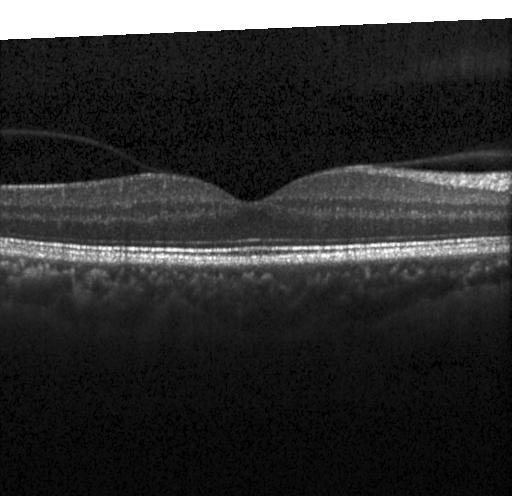 Impression: no evidence of choroidal neovascularization, diabetic macular edema, or drusen.